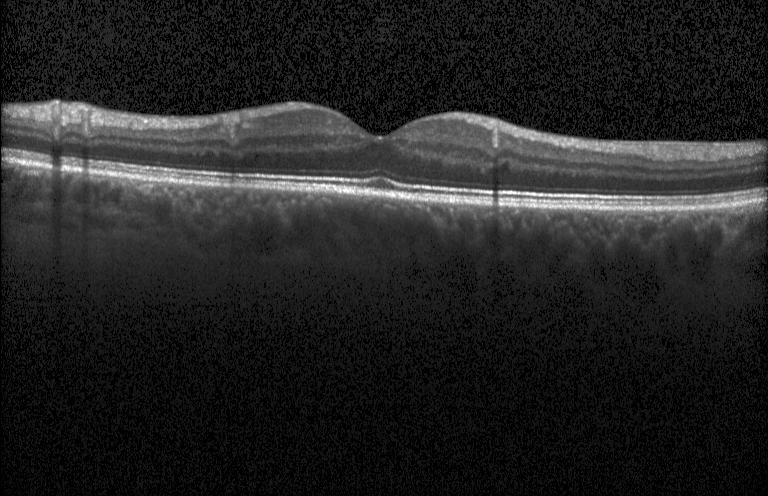 Retinal OCT cross-section. Heidelberg Spectralis. Horizontal scan through the fovea — Finding: no CNV, no DME, and no drusen.